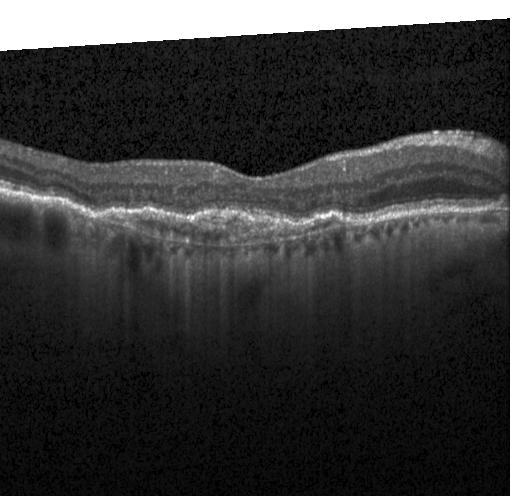 Dx: choroidal neovascularization.